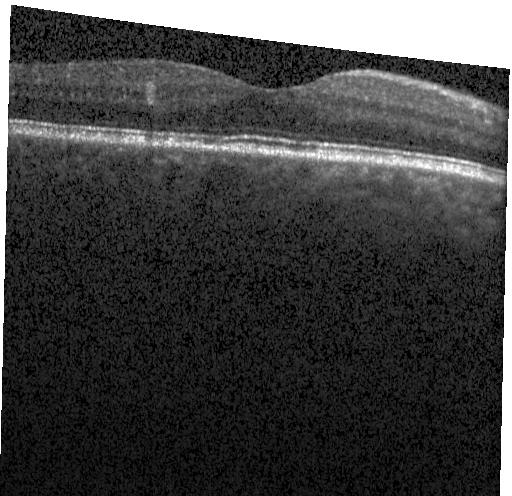 OCT scan showing no CNV, DME, or drusen.